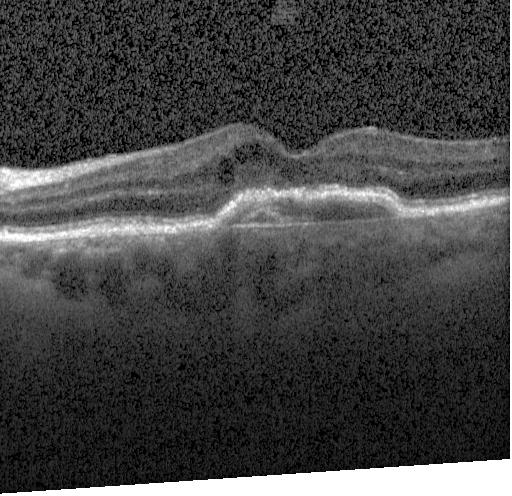 Optical coherence tomography B-scan; through the macula; spectral-domain optical coherence tomography.
The scan shows a choroidal neovascular membrane.